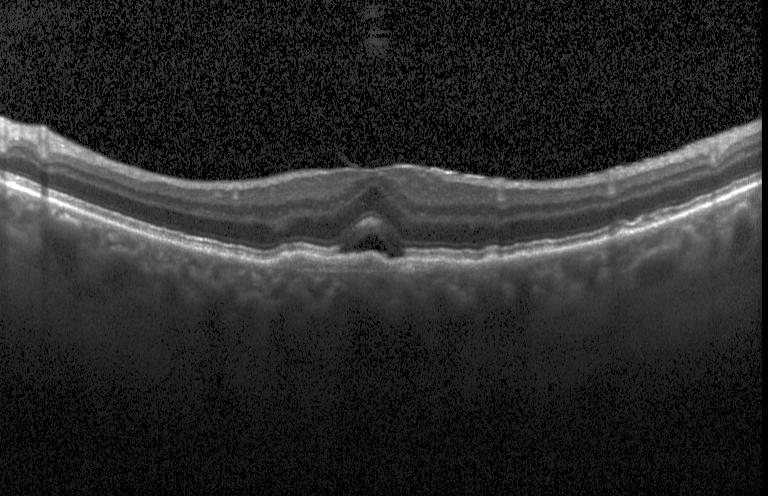

Instrument: Heidelberg Spectralis · optical coherence tomography B-scan.
Macular OCT: a choroidal neovascular membrane.